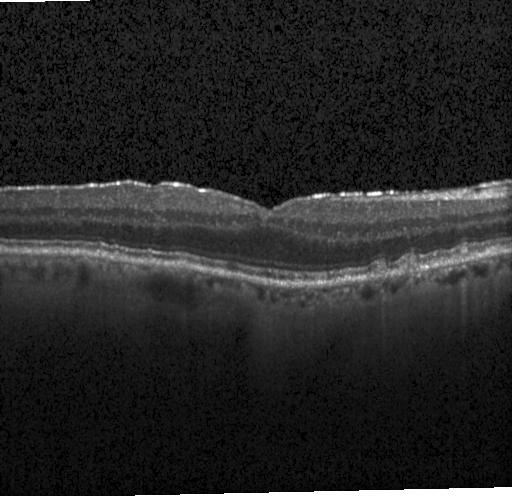

The scan shows drusen.